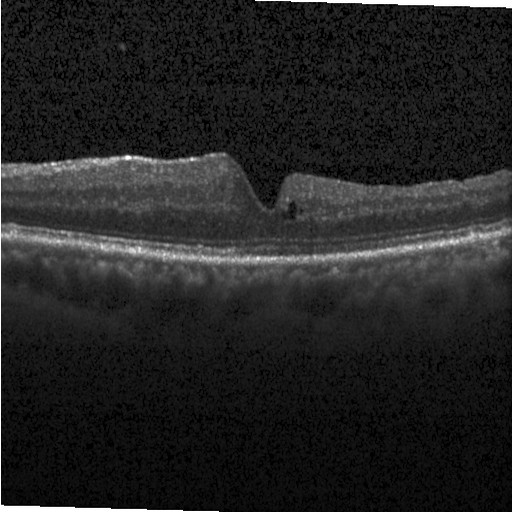 Optical coherence tomography B-scan
Impression: diabetic macular edema (DME).